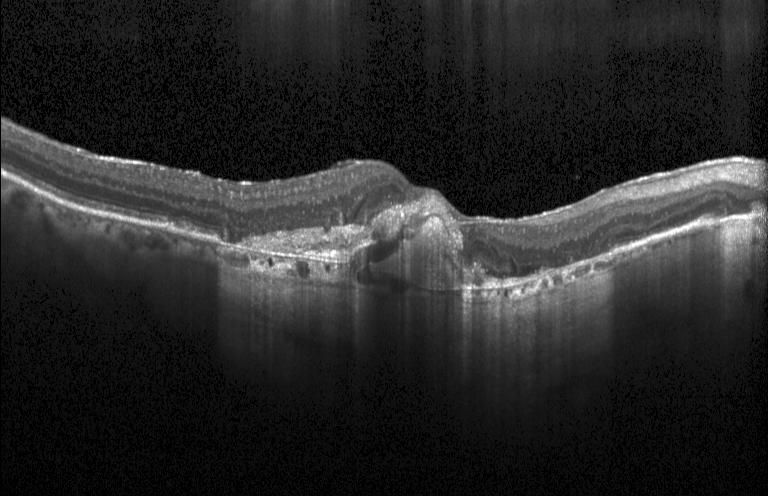

Spectral-domain optical coherence tomography. Retinal OCT B-scan. Heidelberg Spectralis OCT system. Macular scan
Dx: a choroidal neovascular membrane.